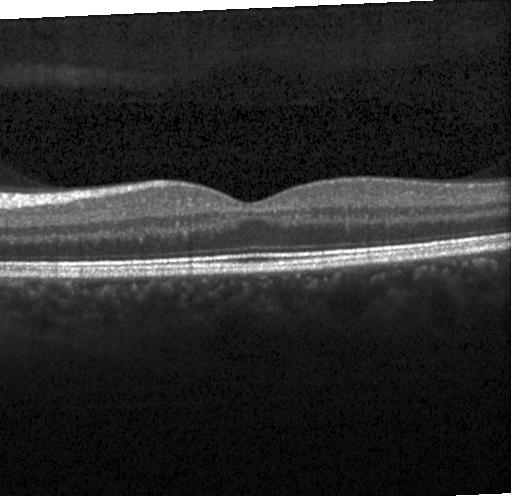

Heidelberg Spectralis OCT system; optical coherence tomography B-scan — This B-scan demonstrates neither choroidal neovascularization, diabetic macular edema, nor drusen.